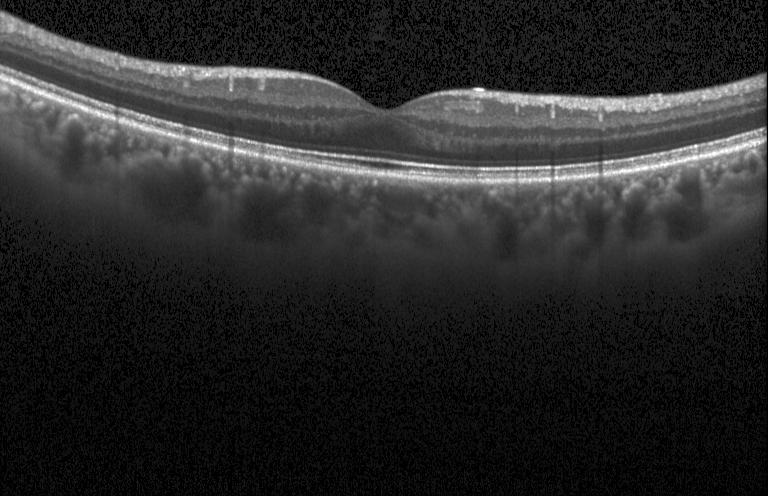 OCT B-scan · spectral-domain optical coherence tomography
The scan shows no choroidal neovascularization, no diabetic macular edema, and no drusen.